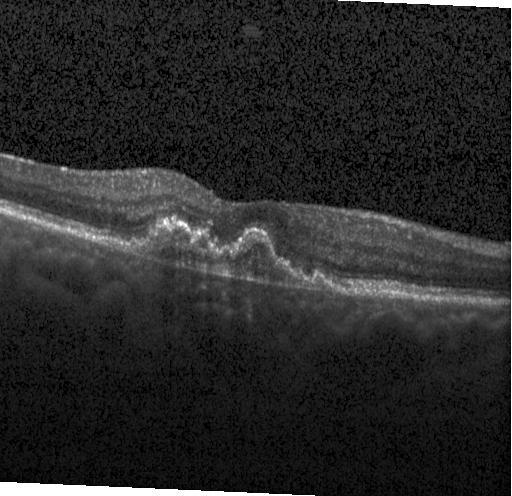
Macular OCT: choroidal neovascularization (CNV).